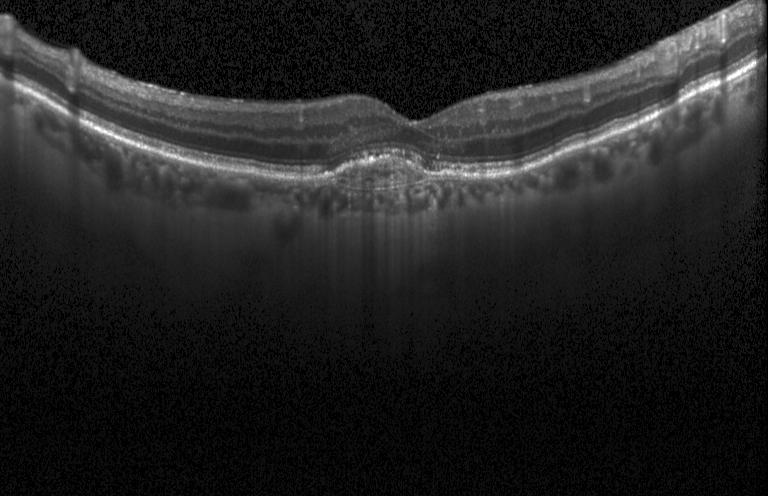
Optical coherence tomography B-scan; spectral-domain optical coherence tomography. Diagnosis: a choroidal neovascular membrane.